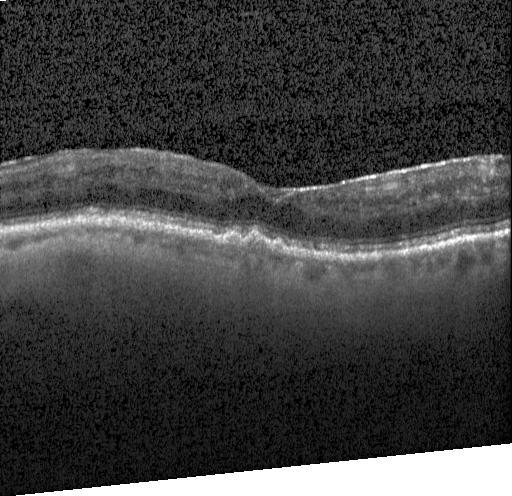
Finding: sub-RPE drusenoid deposits.